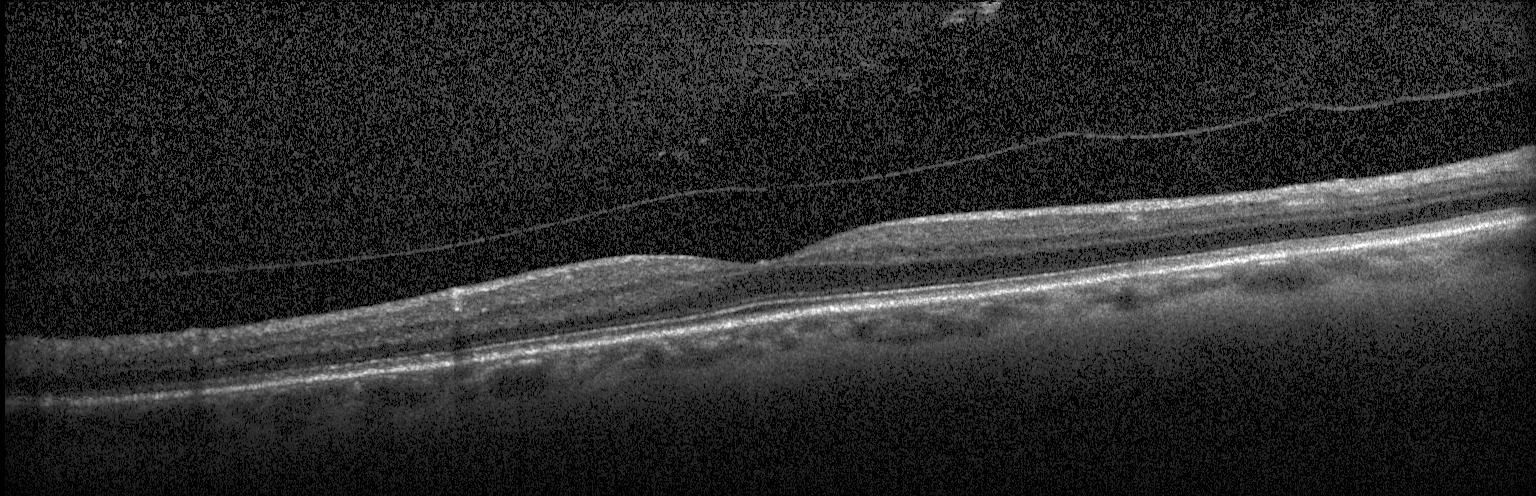
Instrument: Heidelberg Spectralis. SD-OCT. Optical coherence tomography scan. Macular scan — Finding: neither choroidal neovascularization, diabetic macular edema, nor drusen.